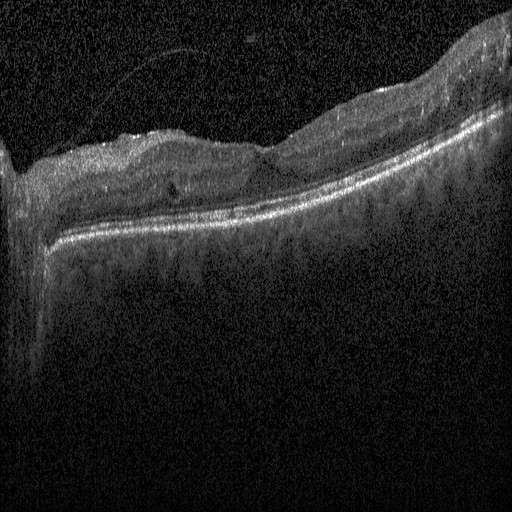

Spectral-domain optical coherence tomography. OCT B-scan. Centered on the fovea
Impression: diabetic macular edema.